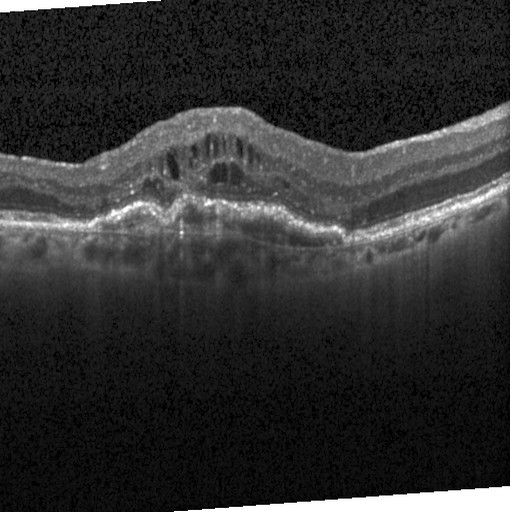

OCT B-scan, SD-OCT, instrument: Heidelberg Spectralis — OCT finding: diabetic macular edema (DME).